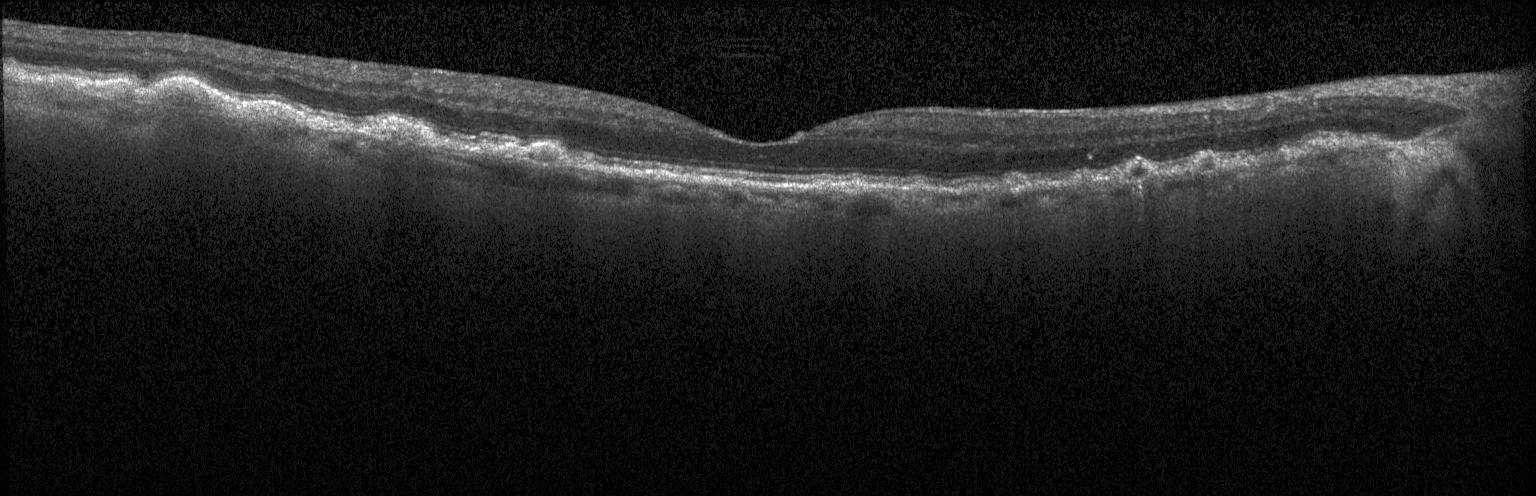

Multiple drusen.